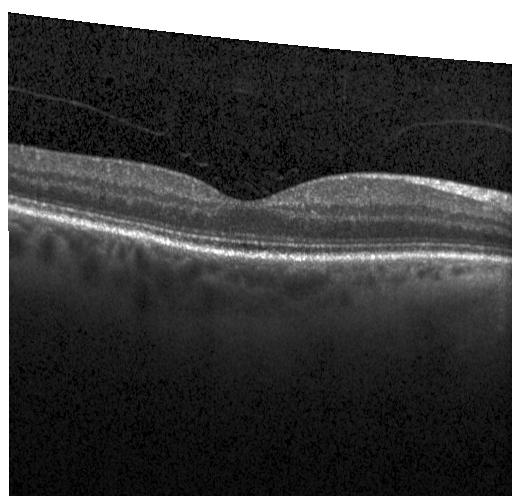

Retinal OCT B-scan
Diagnosis: neither choroidal neovascularization, diabetic macular edema, nor drusen.